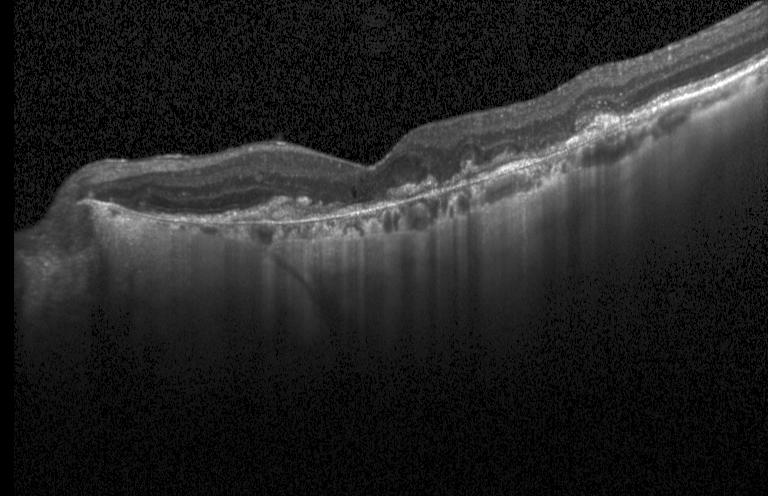 OCT B-scan; SD-OCT; horizontal scan through the fovea. Assessment: a choroidal neovascular membrane.